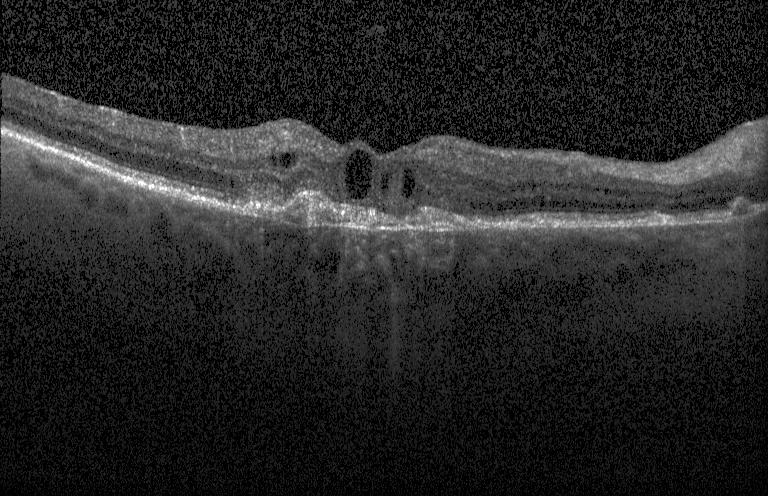
Fovea-centered. Optical coherence tomography B-scan
Diagnosis: a choroidal neovascular membrane.